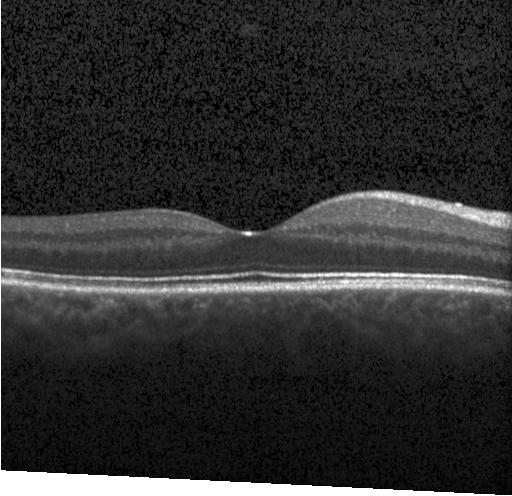

Spectral-domain OCT B-scan: neither choroidal neovascularization, diabetic macular edema, nor drusen.